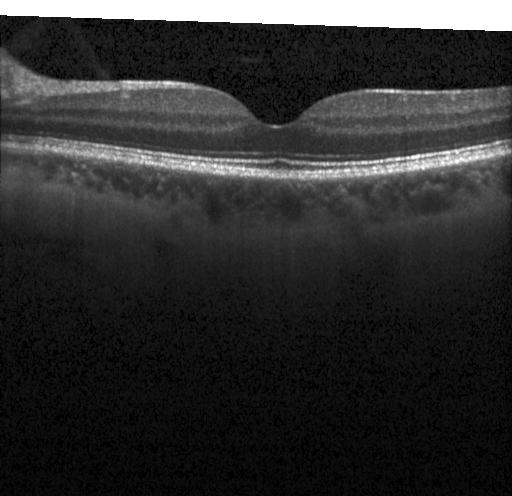

Optical coherence tomography B-scan.
OCT finding: neither choroidal neovascularization, diabetic macular edema, nor drusen.